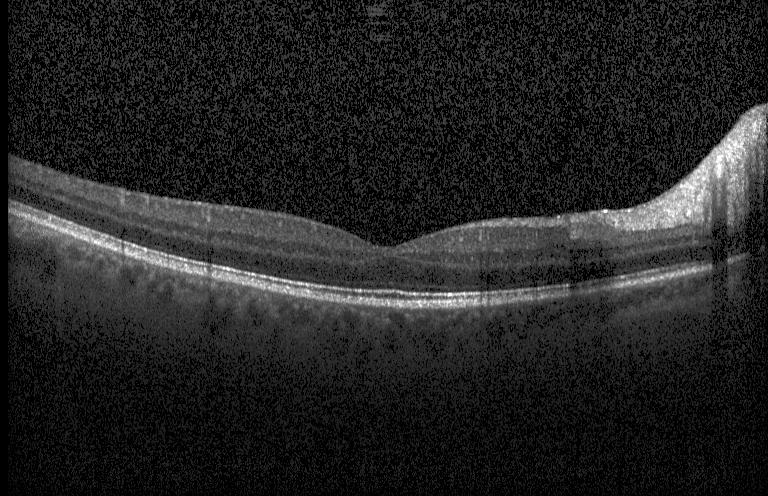 OCT B-scan showing neither CNV, DME, nor drusen.